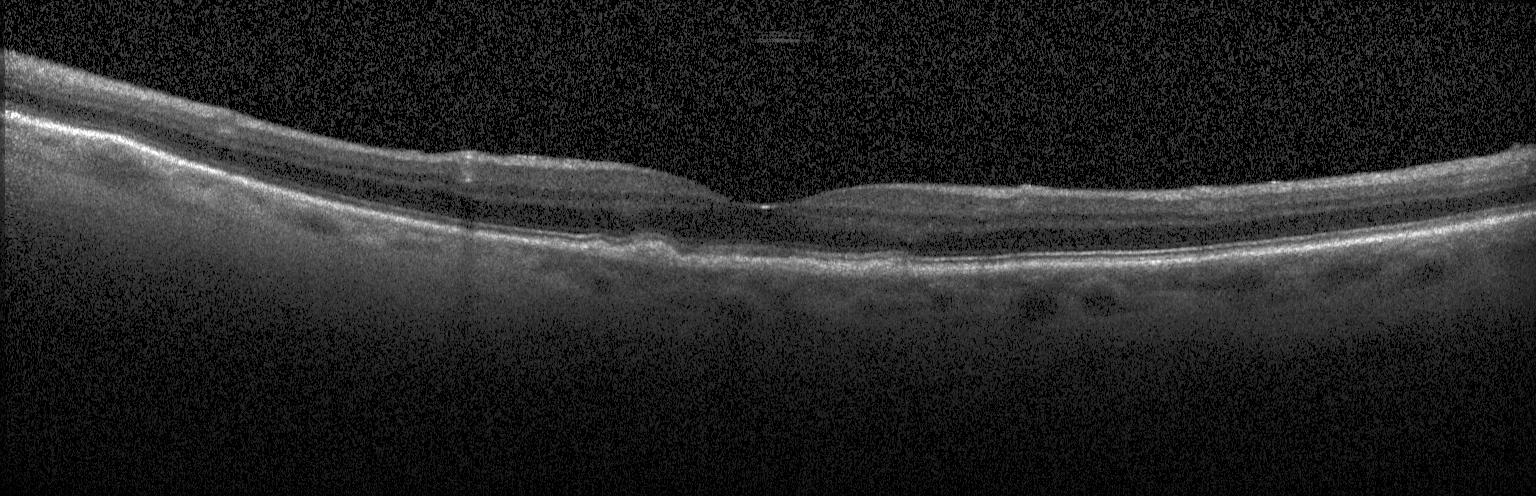
OCT B-scan. SD-OCT. Acquired on a Heidelberg Spectralis — This B-scan demonstrates sub-RPE drusenoid deposits.